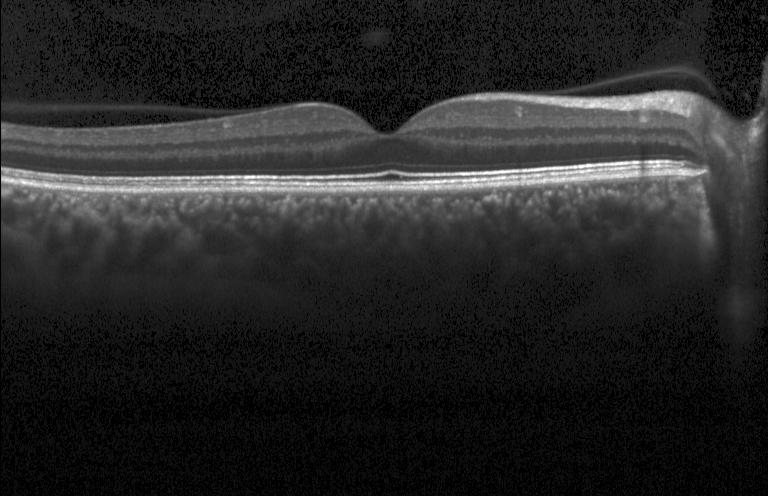
Optical coherence tomography B-scan — OCT finding: no CNV, DME, or drusen.